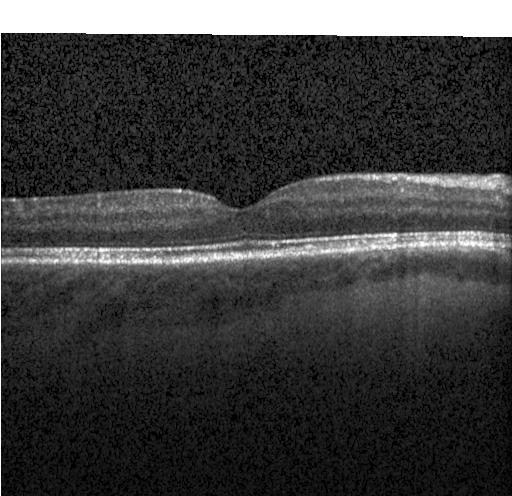

Spectral-domain optical coherence tomography. Retinal OCT B-scan. Macular scan
The scan shows no evidence of choroidal neovascularization, diabetic macular edema, or drusen.